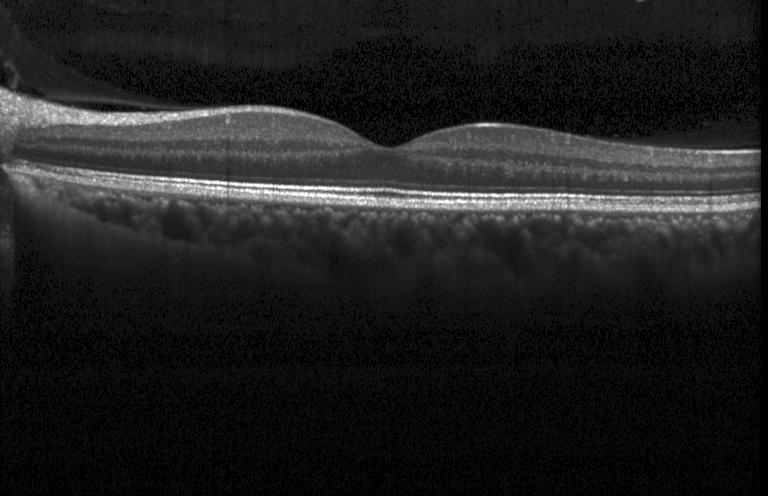
SD-OCT; optical coherence tomography B-scan; fovea-centered; acquired on a Heidelberg Spectralis — Dx: no choroidal neovascularization, no diabetic macular edema, and no drusen.